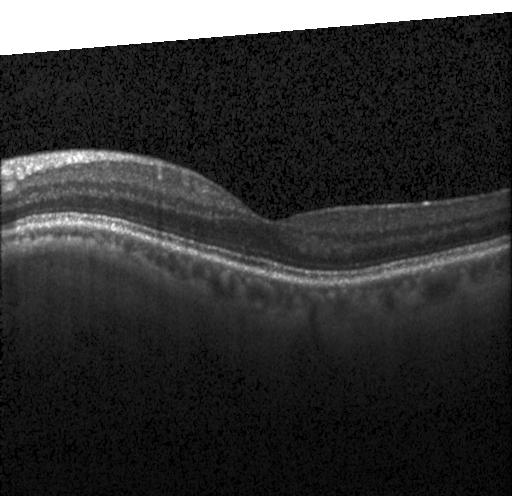
Assessment: no evidence of choroidal neovascularization, diabetic macular edema, or drusen.